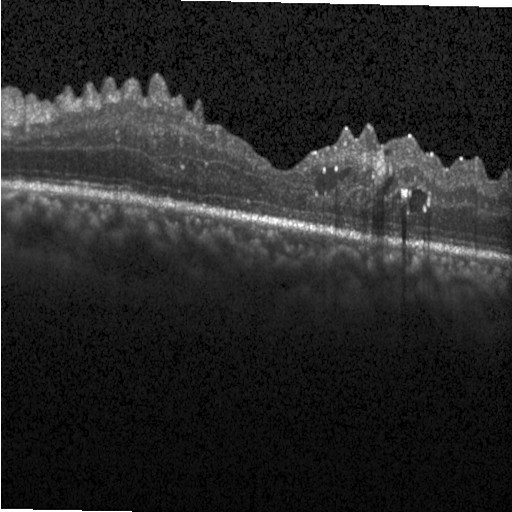

Horizontal scan through the fovea. OCT B-scan
Finding: diabetic macular edema (DME).